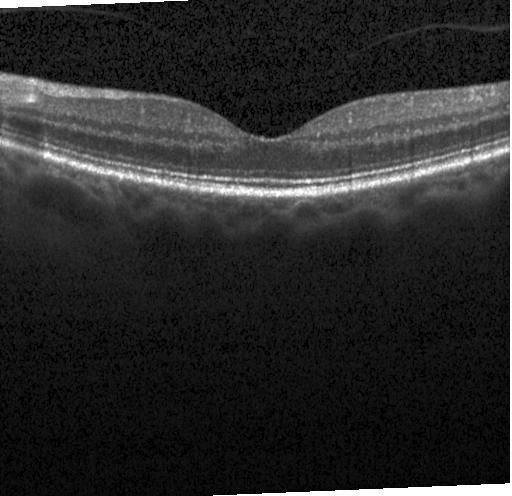

Fovea-centered, optical coherence tomography B-scan, acquired on a Heidelberg Spectralis
OCT finding: neither choroidal neovascularization, diabetic macular edema, nor drusen.